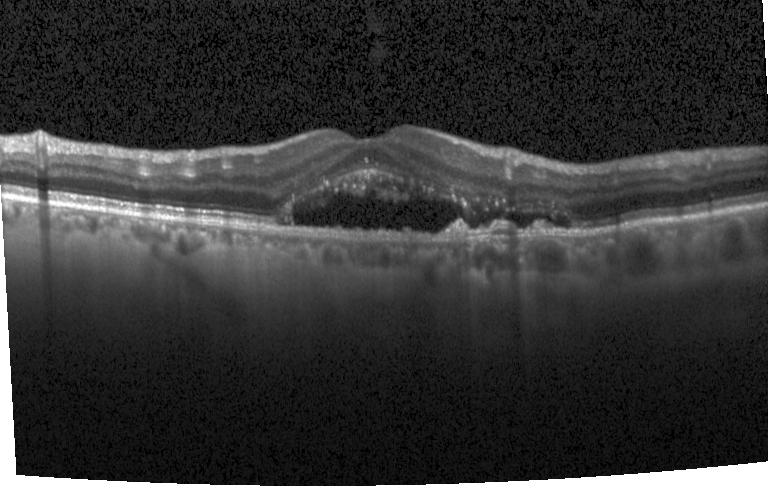 Diagnosis: choroidal neovascularization (CNV).